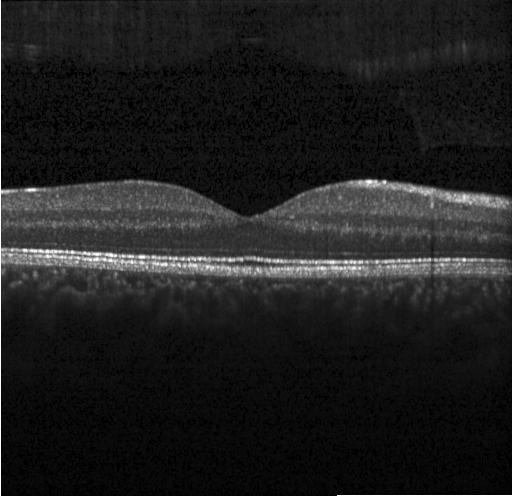 Retinal OCT cross-section showing no choroidal neovascularization, no diabetic macular edema, and no drusen.